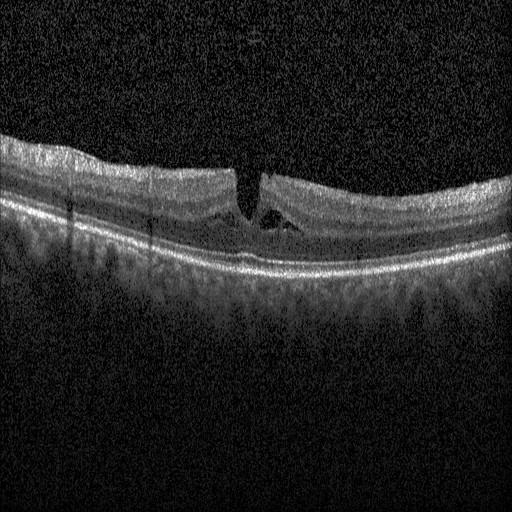 Retinal OCT B-scan · instrument: Heidelberg Spectralis · macular scan
Finding: DME.